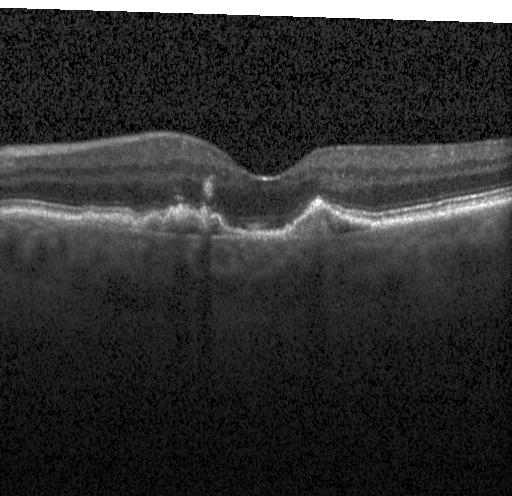 Dx: choroidal neovascularization.